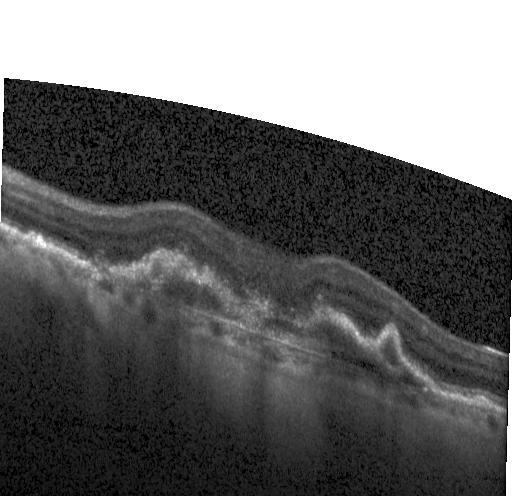

Retinal OCT cross-section. Through the macula.
Finding: choroidal neovascularization (CNV).